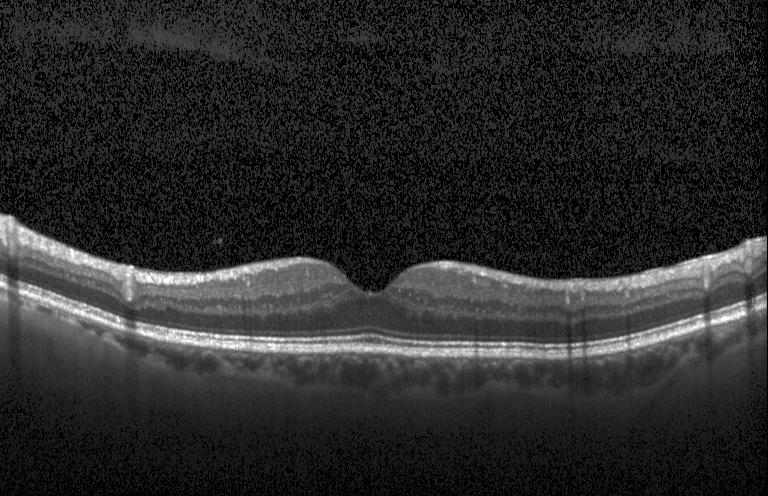

Retinal OCT B-scan · through the macula · spectral-domain optical coherence tomography. Macular OCT: neither choroidal neovascularization, diabetic macular edema, nor drusen.